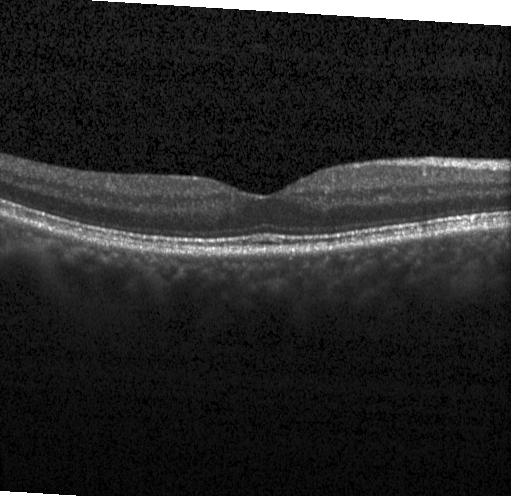 Retinal OCT B-scan.
The scan shows no evidence of choroidal neovascularization, diabetic macular edema, or drusen.